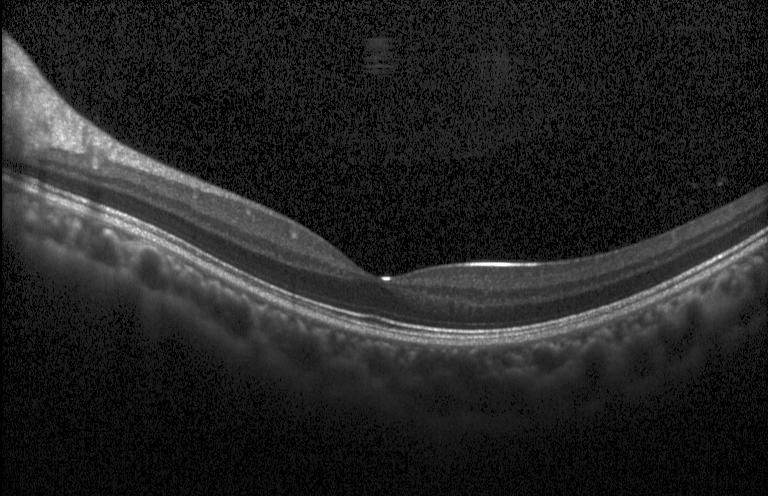 Optical coherence tomography B-scan
Assessment: neither CNV, DME, nor drusen.